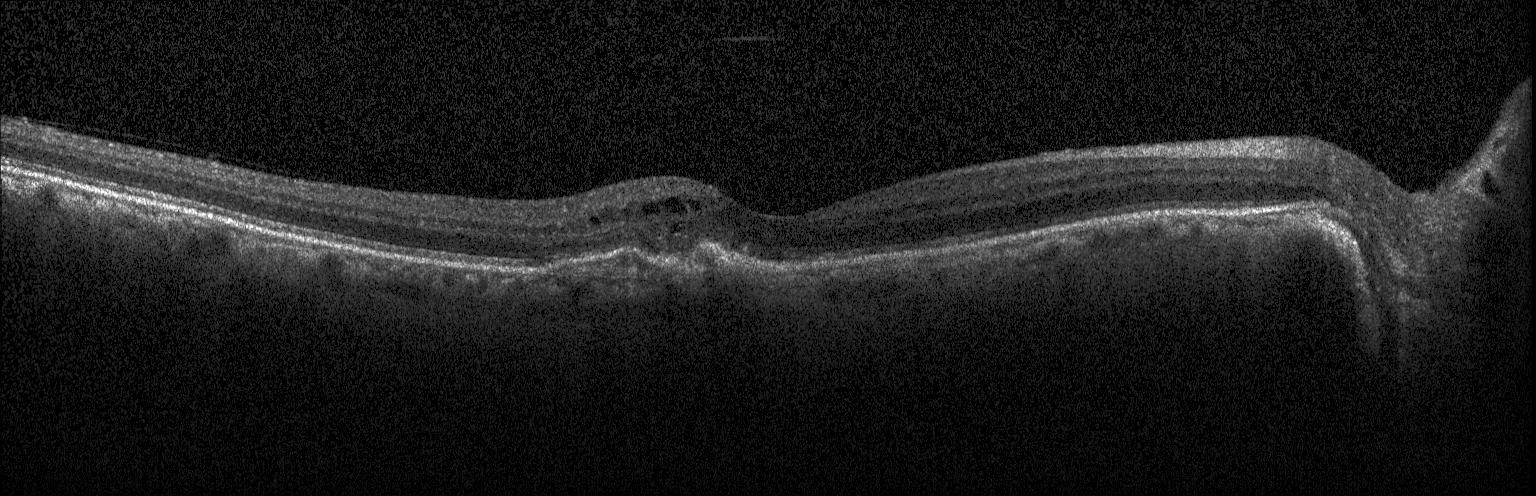

Diagnosis: choroidal neovascularization.